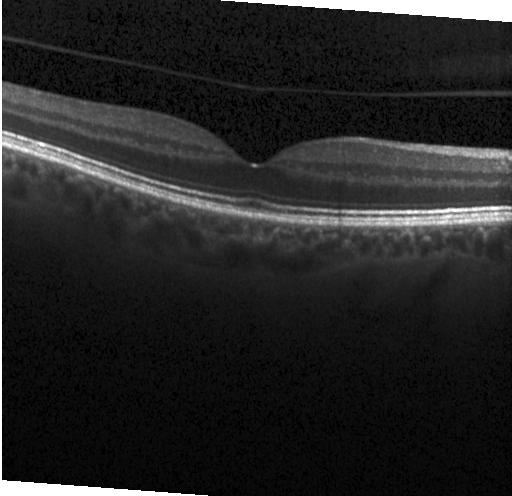 OCT B-scan. Finding: no choroidal neovascularization, diabetic macular edema, or drusen.